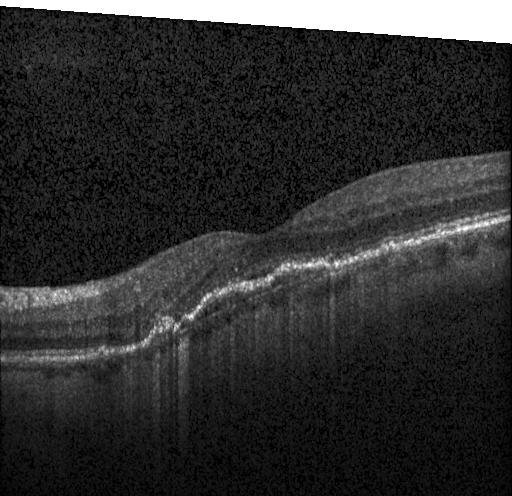
OCT line scan
Finding: choroidal neovascularization.